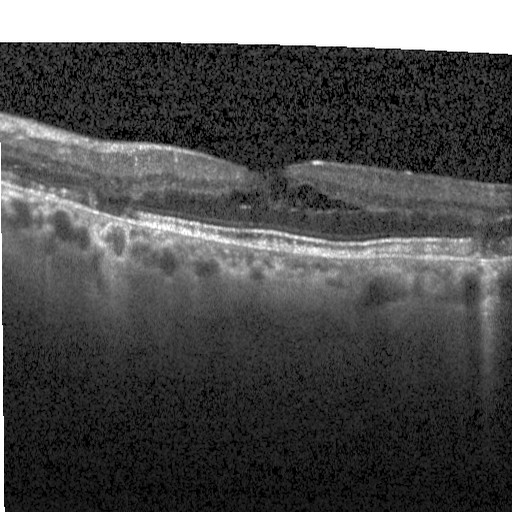 Optical coherence tomography scan.
Finding: diabetic macular edema (DME).